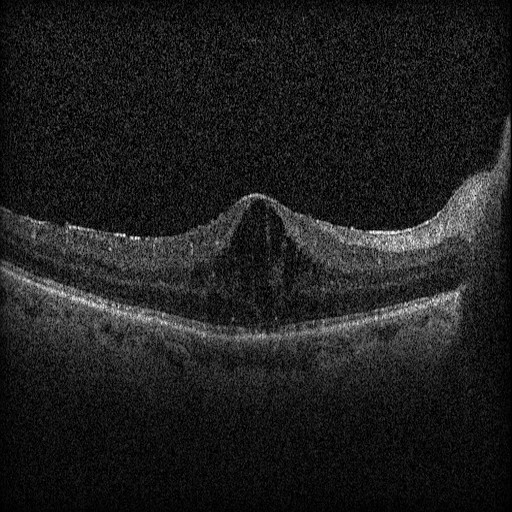
Diagnosis: diabetic macular edema.